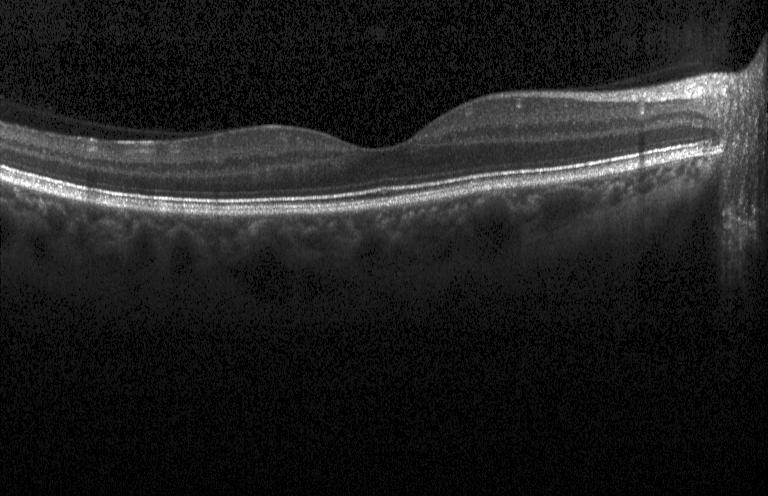 No choroidal neovascularization, no diabetic macular edema, and no drusen.